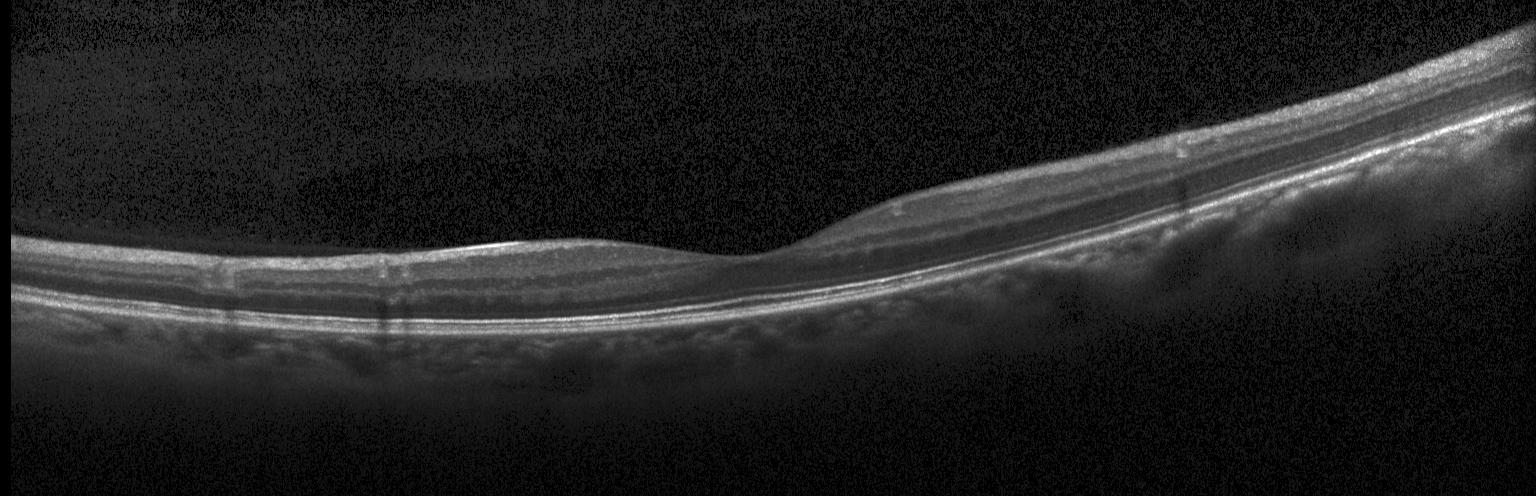
Centered on the fovea. OCT line scan. Heidelberg Spectralis — This B-scan demonstrates no choroidal neovascularization, diabetic macular edema, or drusen.